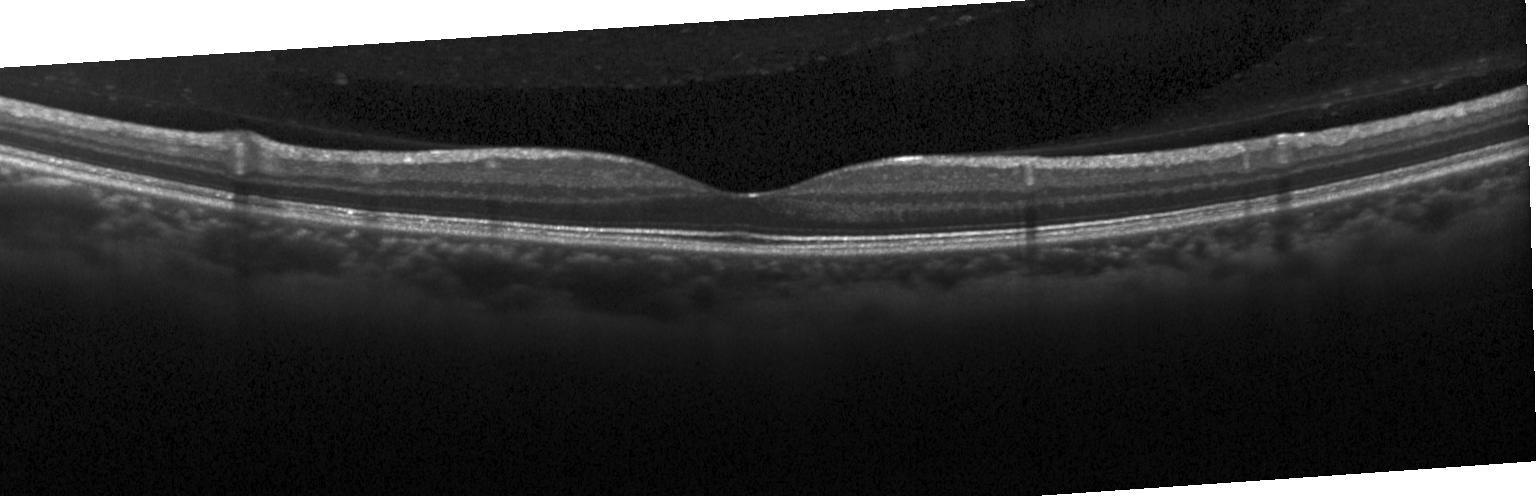
Optical coherence tomography B-scan · spectral-domain optical coherence tomography
Neither CNV, DME, nor drusen.